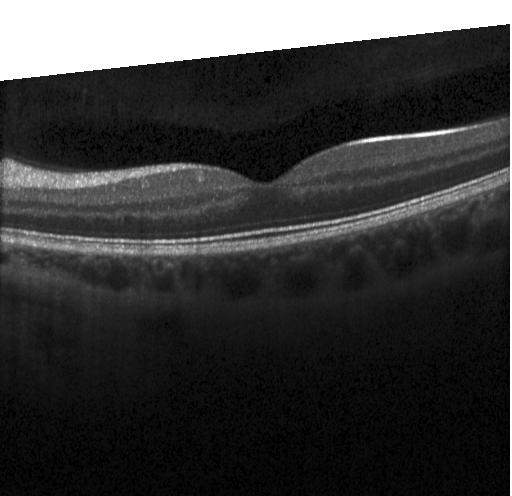
Retinal OCT B-scan
Finding: neither choroidal neovascularization, diabetic macular edema, nor drusen.